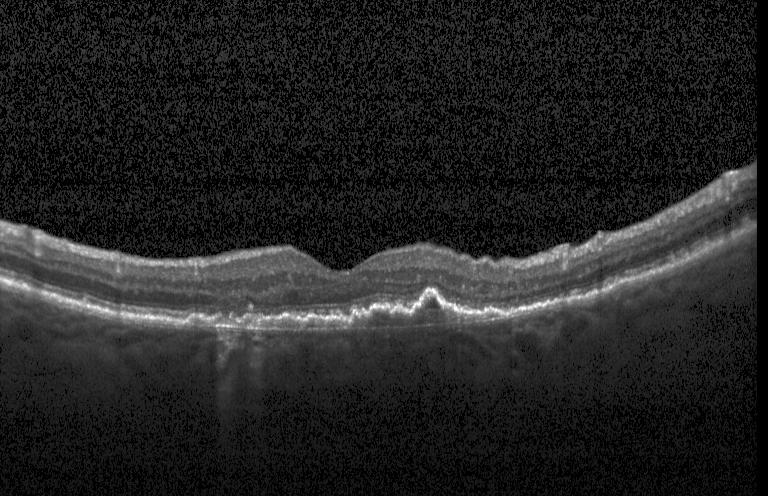
Optical coherence tomography scan; instrument: Heidelberg Spectralis — Impression: CNV.